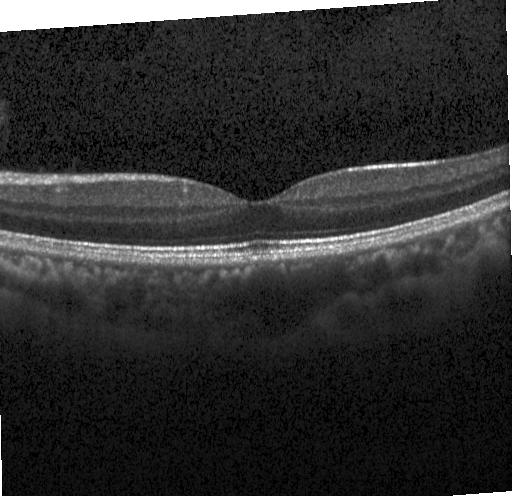

SD-OCT, retinal OCT cross-section, instrument: Heidelberg Spectralis
OCT finding: neither choroidal neovascularization, diabetic macular edema, nor drusen.